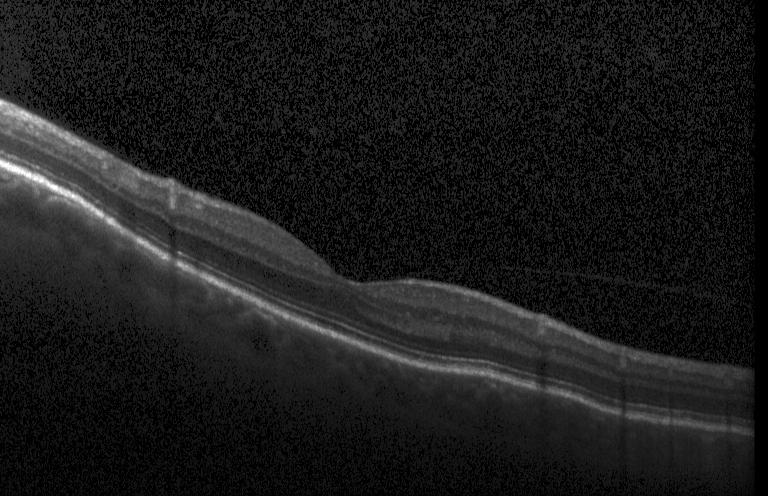 Diagnosis: no choroidal neovascularization, no diabetic macular edema, and no drusen.